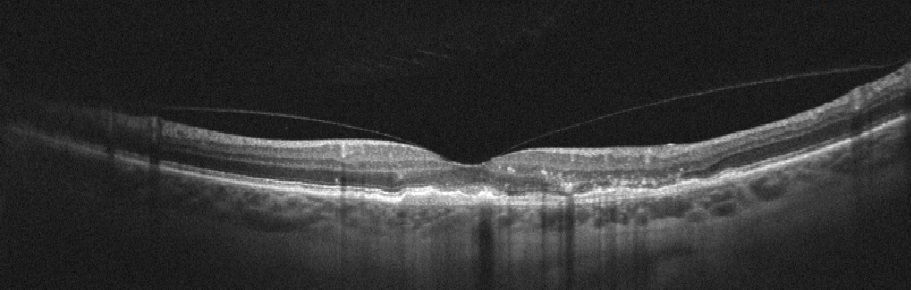

Optical coherence tomography scan · macular scan · acquired on an Optovue Avanti RTVue XR. Finding: AMD.